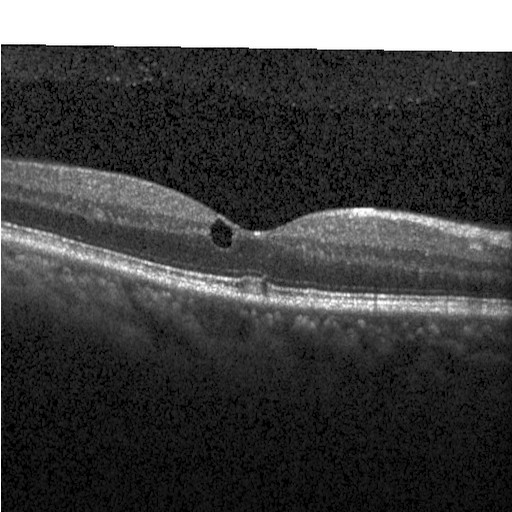

Retinal OCT B-scan · spectral-domain optical coherence tomography · Heidelberg Spectralis OCT system
This B-scan demonstrates DME.